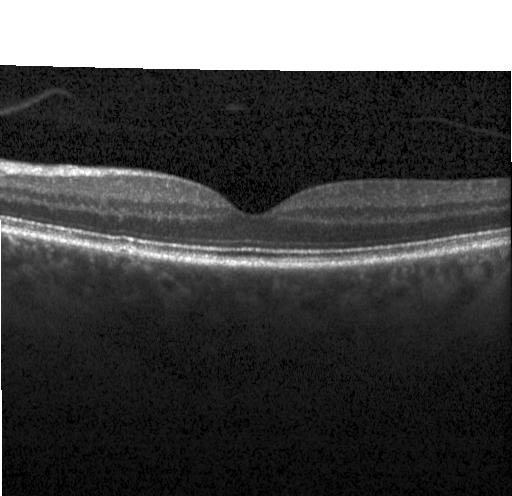 Retinal OCT cross-section showing no evidence of choroidal neovascularization, diabetic macular edema, or drusen.